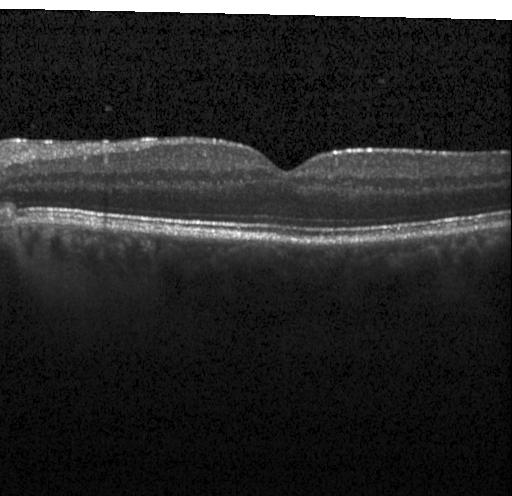 Spectral-domain OCT B-scan: no choroidal neovascularization, no diabetic macular edema, and no drusen.